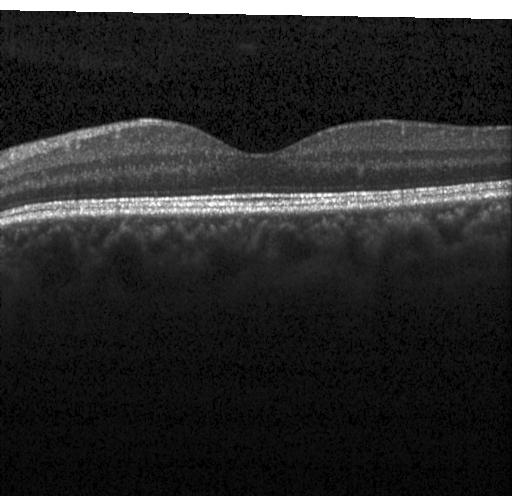 Fovea-centered, OCT B-scan, instrument: Heidelberg Spectralis, spectral-domain OCT
Finding: no evidence of choroidal neovascularization, diabetic macular edema, or drusen.